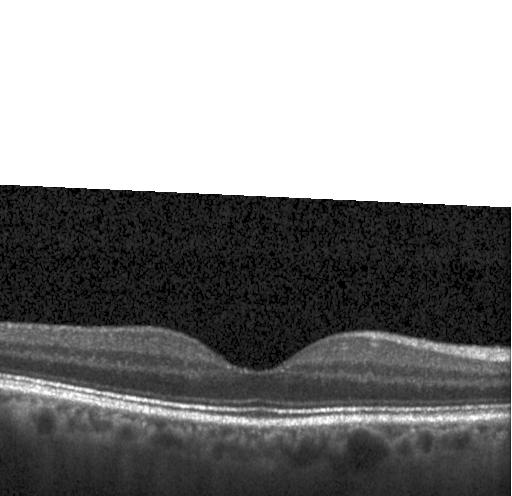 Retinal OCT B-scan
OCT finding: no CNV, DME, or drusen.